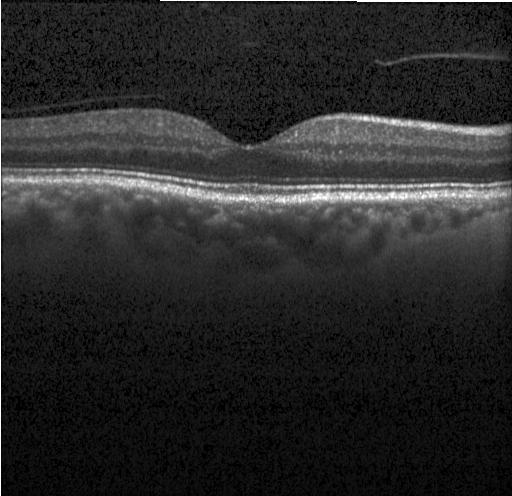
Spectral-domain OCT B-scan: no choroidal neovascularization, diabetic macular edema, or drusen.